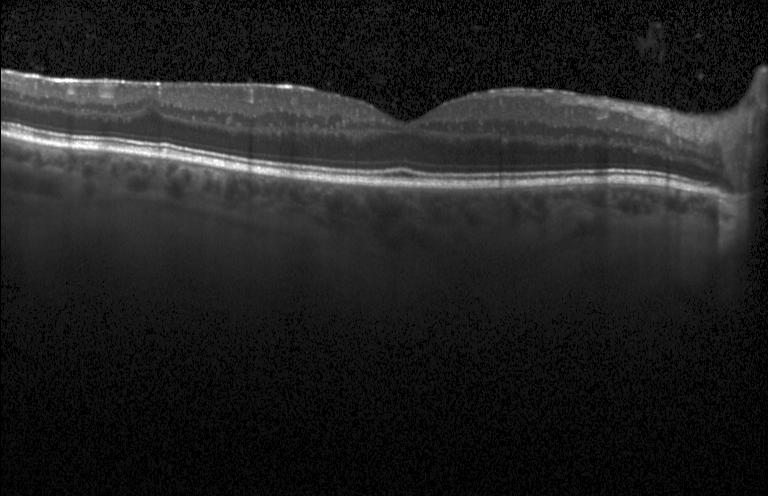 Centered on the fovea, OCT B-scan, spectral-domain optical coherence tomography, acquired on a Heidelberg Spectralis — Finding: no CNV, no DME, and no drusen.